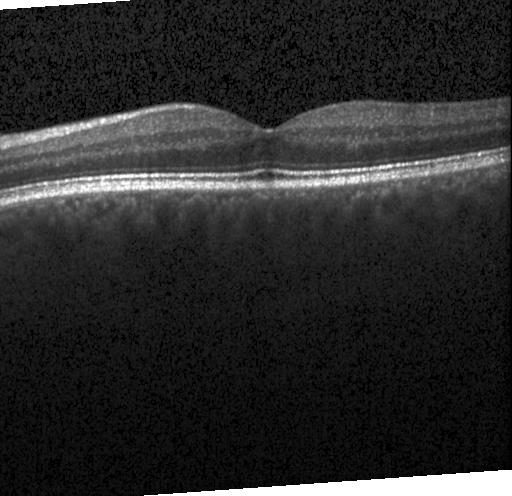
OCT finding: no evidence of CNV, DME, or drusen.